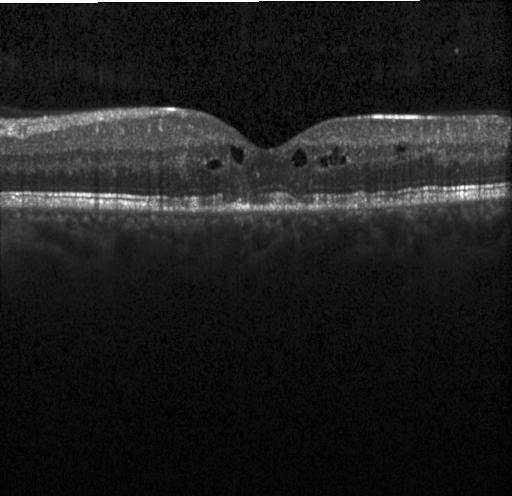 Heidelberg Spectralis; OCT B-scan. Finding: diabetic macular edema (DME).